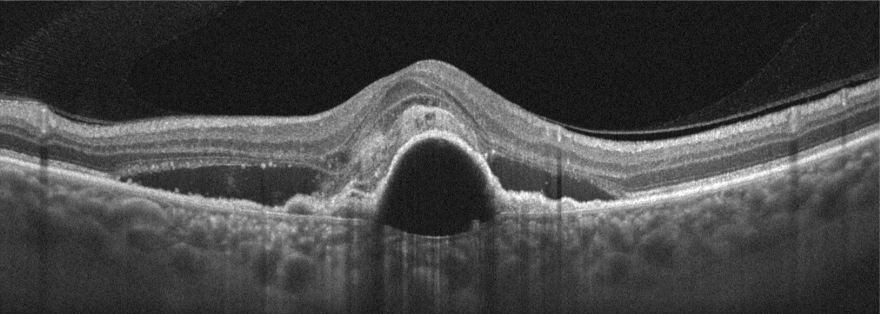 Impression: age-related macular degeneration (AMD).